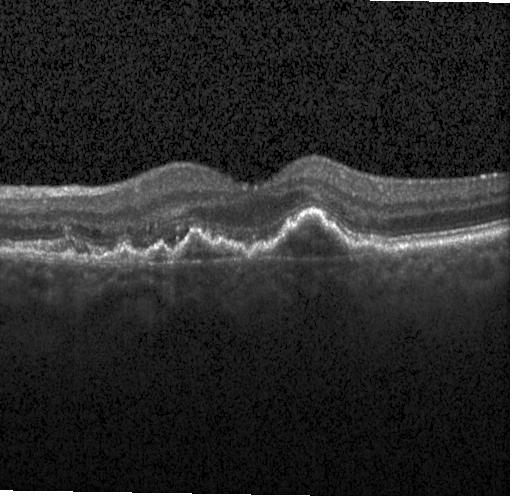

Retinal OCT cross-section showing CNV.